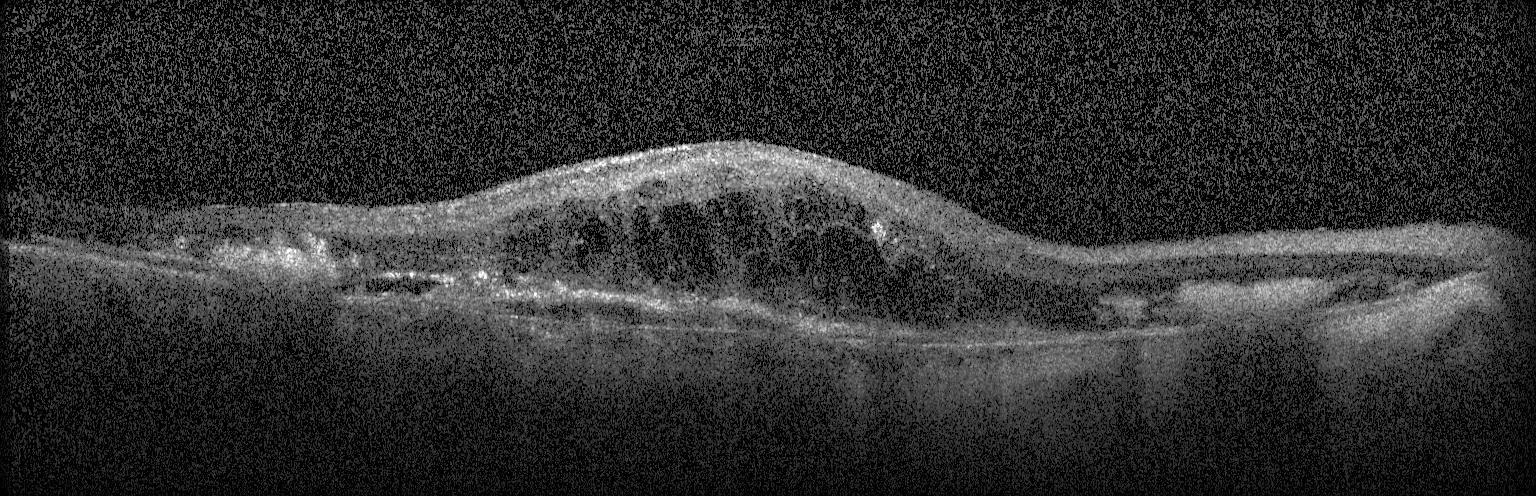

This B-scan demonstrates CNV.